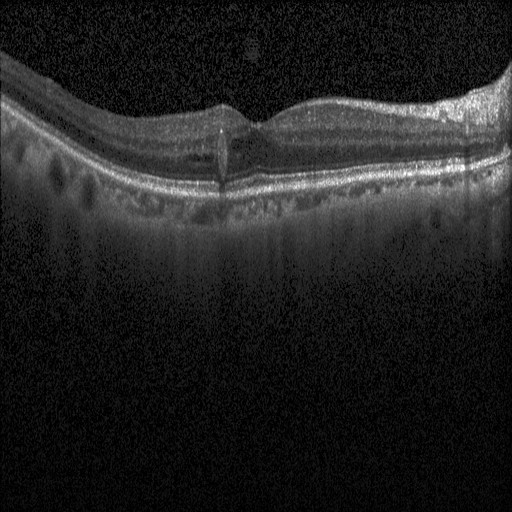

Diagnosis: diabetic macular edema (DME).